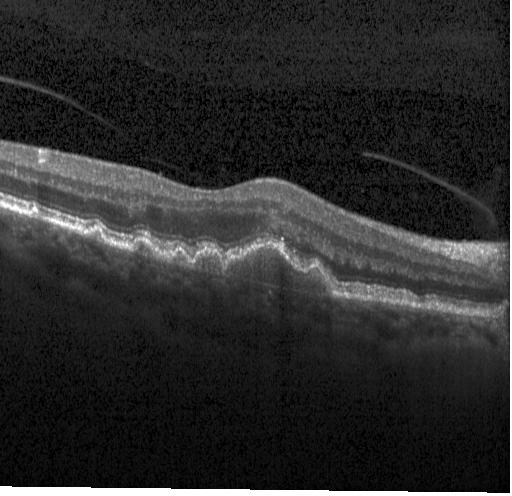
Macular scan. Acquired on a Heidelberg Spectralis. Optical coherence tomography scan. SD-OCT. OCT finding: CNV.